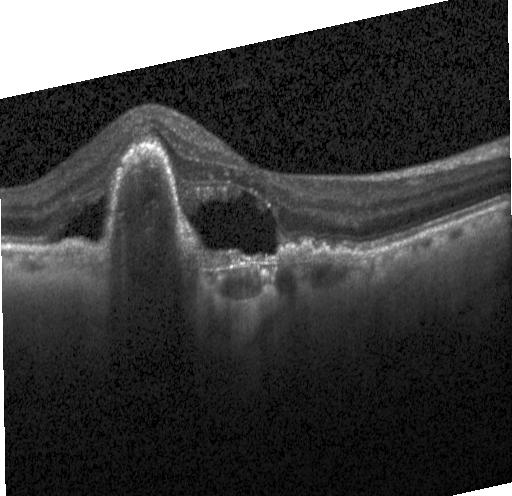

The scan shows a choroidal neovascular membrane.